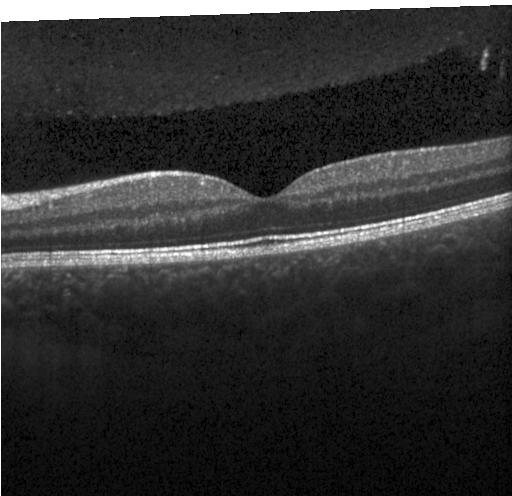
OCT B-scan · SD-OCT · macular scan. Diagnosis: neither choroidal neovascularization, diabetic macular edema, nor drusen.